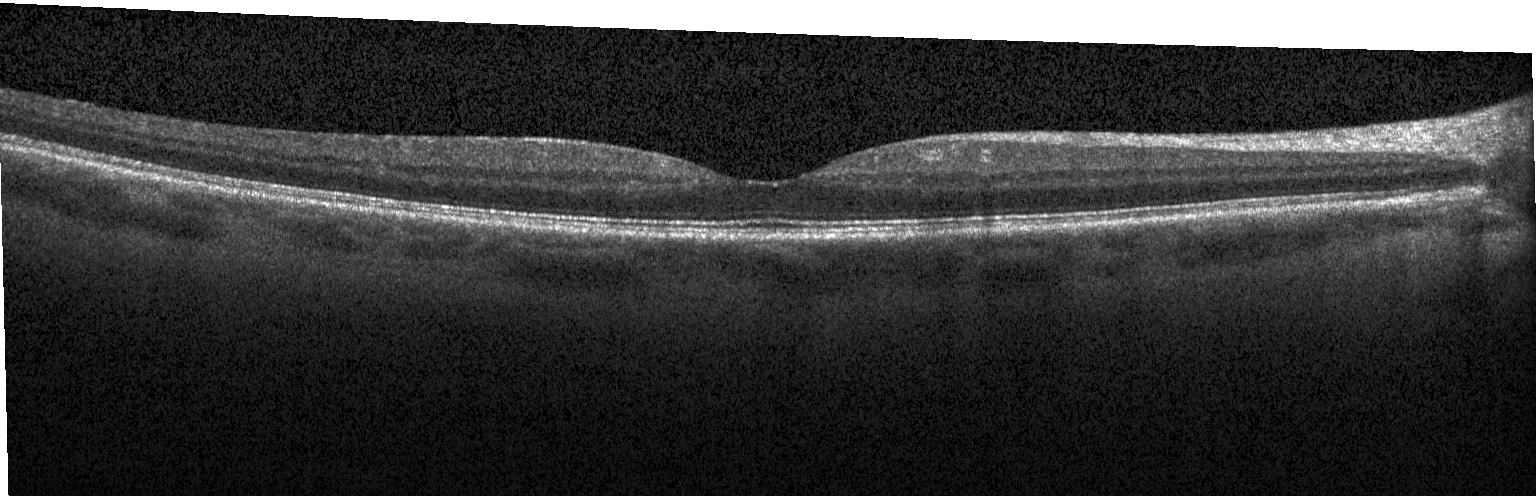
Diagnosis: neither choroidal neovascularization, diabetic macular edema, nor drusen.